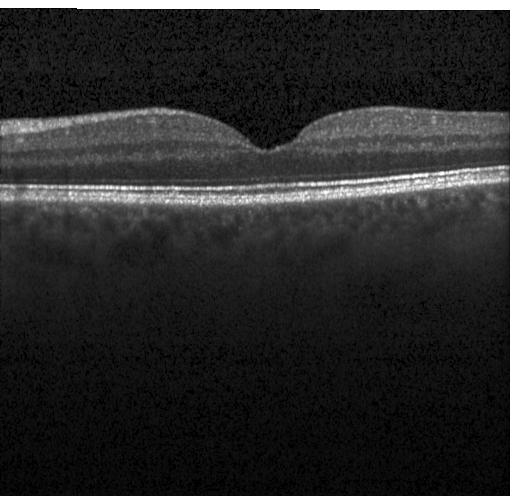

Spectral-domain optical coherence tomography · acquired on a Heidelberg Spectralis · OCT B-scan · fovea-centered.
The scan shows no CNV, no DME, and no drusen.